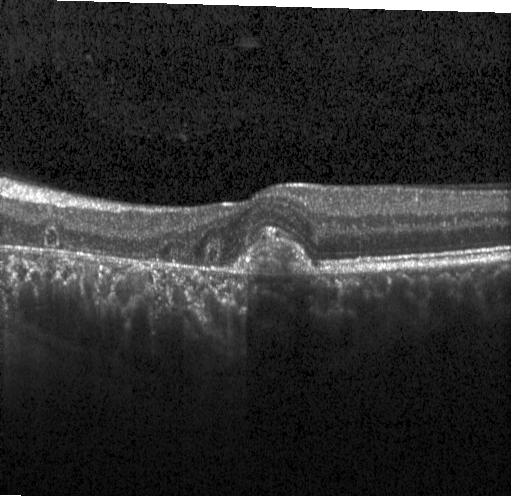

Instrument: Heidelberg Spectralis · horizontal scan through the fovea · SD-OCT · optical coherence tomography scan.
Dx: a choroidal neovascular membrane.